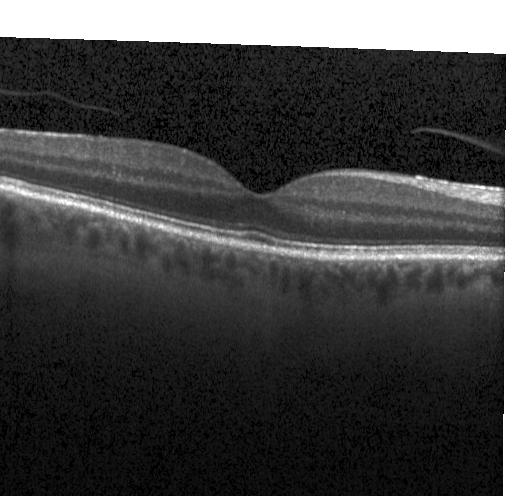
Macular scan · retinal OCT cross-section · spectral-domain optical coherence tomography. Diagnosis: no CNV, DME, or drusen.